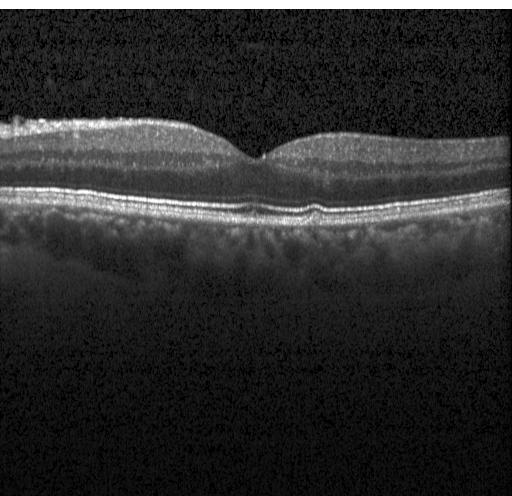
Spectral-domain optical coherence tomography. Acquired on a Heidelberg Spectralis. OCT B-scan
Assessment: drusen.